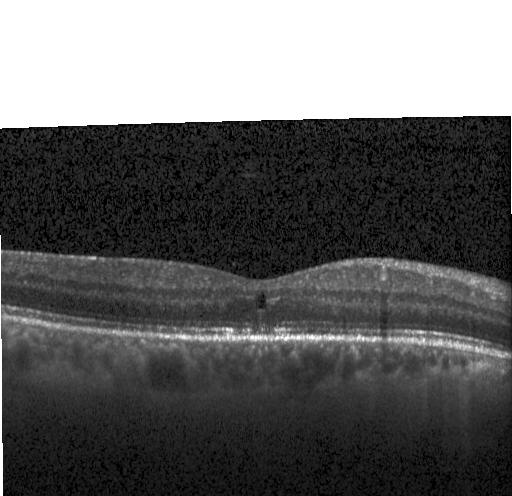
Optical coherence tomography scan. Instrument: Heidelberg Spectralis. Diagnosis: diabetic macular edema.